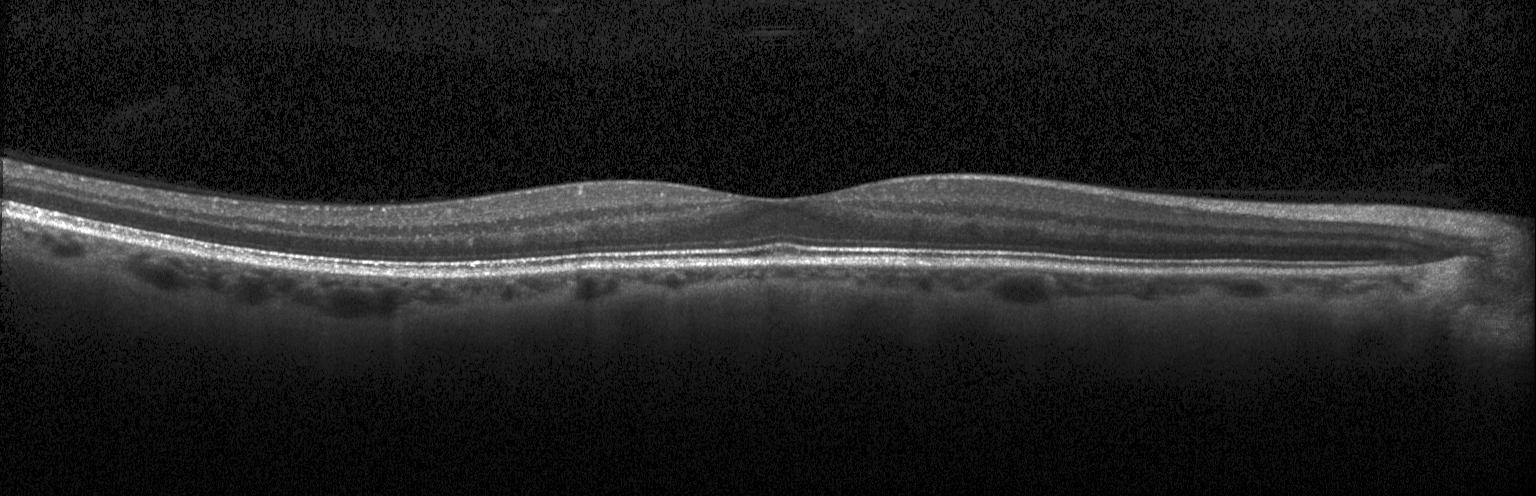 Impression: no CNV, DME, or drusen.